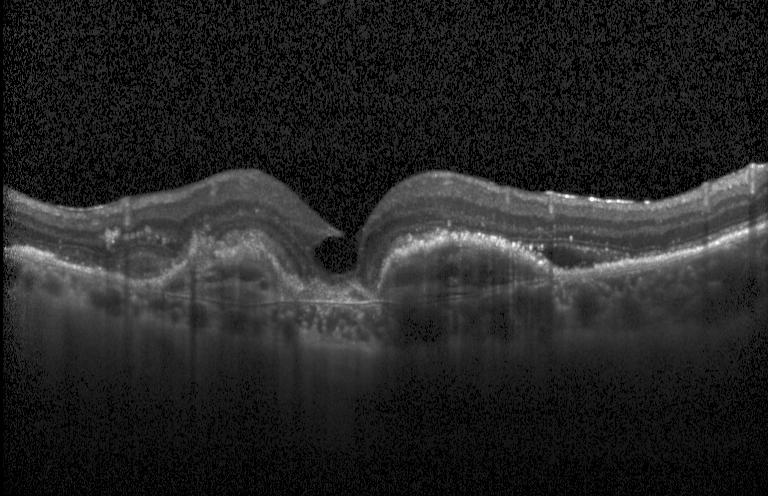

OCT B-scan; spectral-domain optical coherence tomography
OCT finding: a choroidal neovascular membrane.